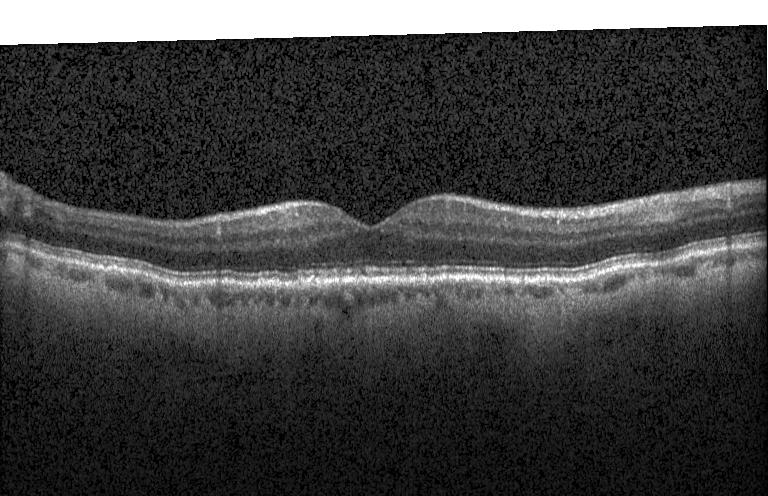 Optical coherence tomography scan — Diagnosis: neither CNV, DME, nor drusen.